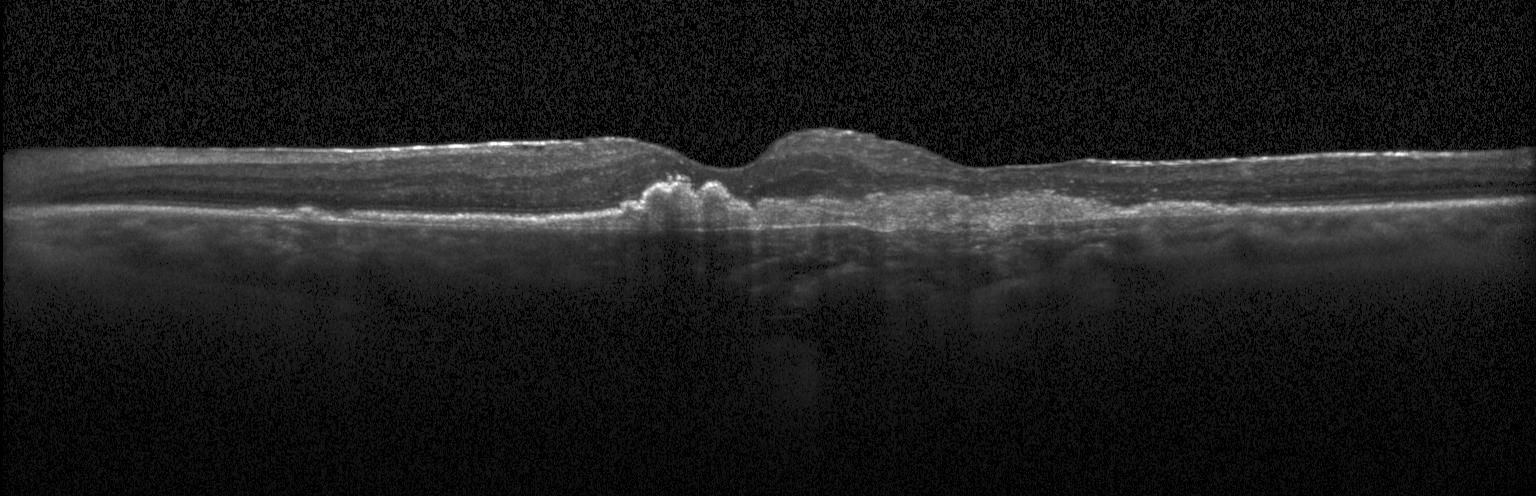
OCT line scan. A choroidal neovascular membrane.